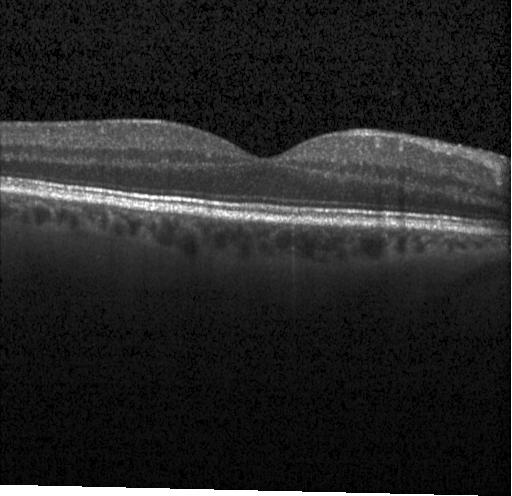 OCT finding: neither choroidal neovascularization, diabetic macular edema, nor drusen.